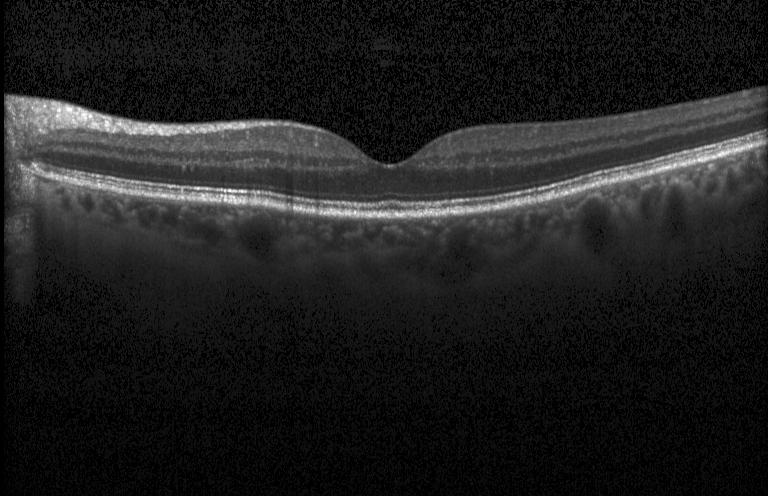 Spectral-domain OCT; retinal OCT cross-section — Finding: no evidence of CNV, DME, or drusen.